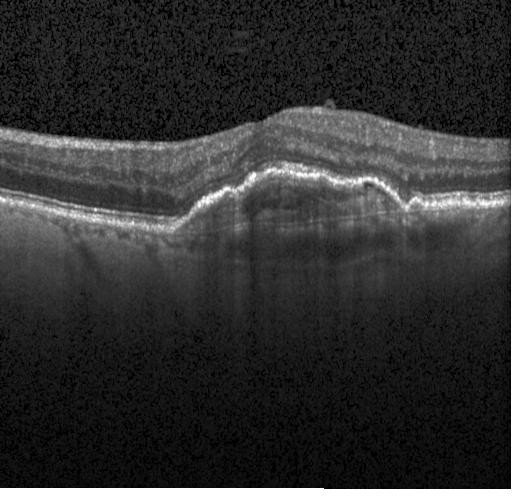

Finding: choroidal neovascularization (CNV).